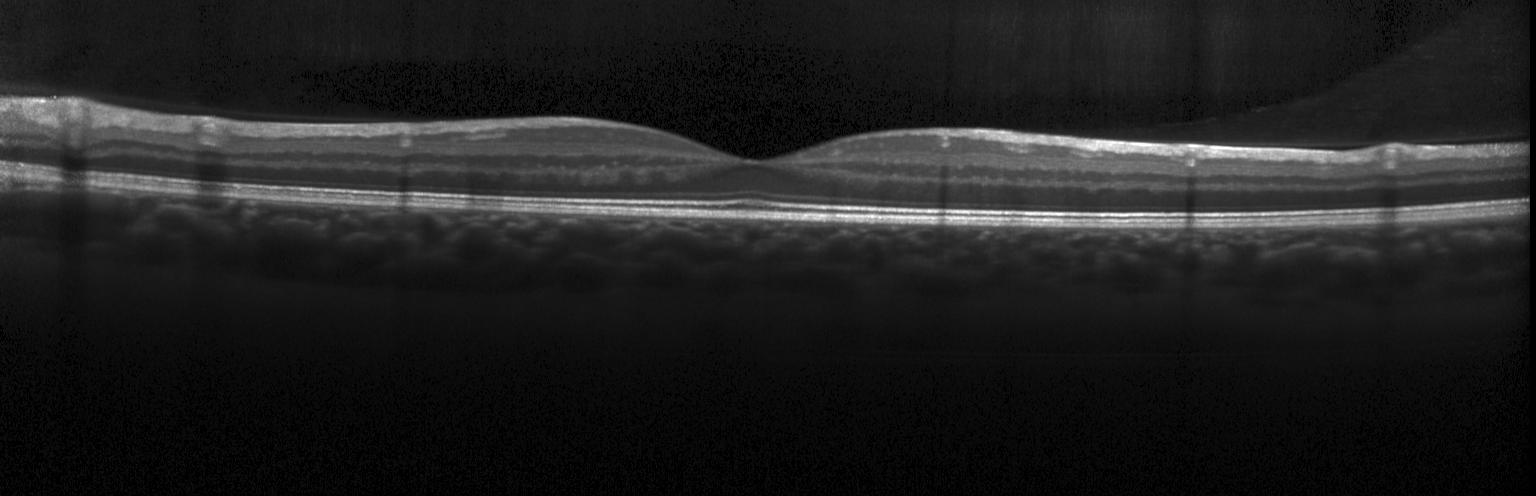

Diagnosis: neither choroidal neovascularization, diabetic macular edema, nor drusen.